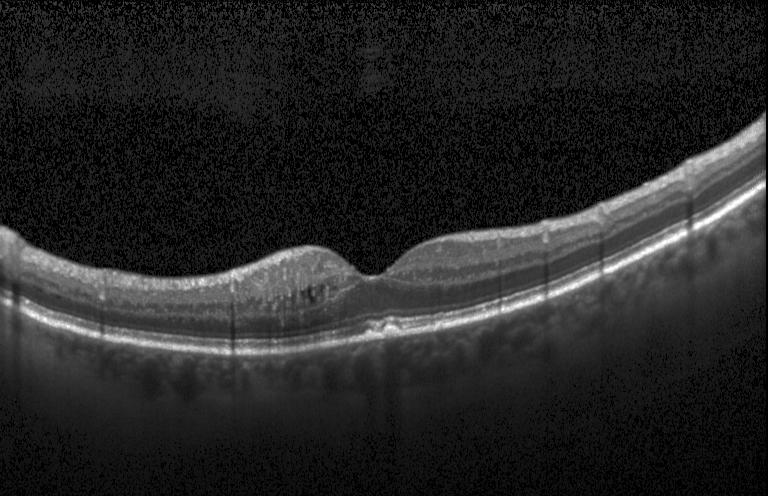 This B-scan demonstrates multiple drusen.